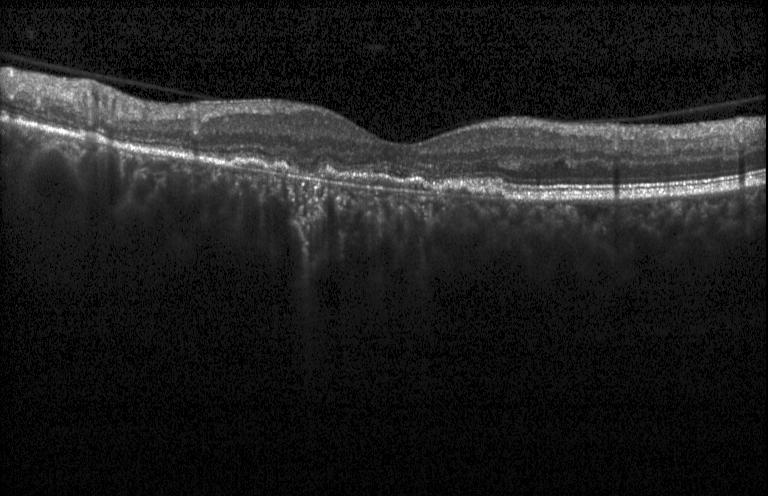

Retinal OCT cross-section — Choroidal neovascularization (CNV).